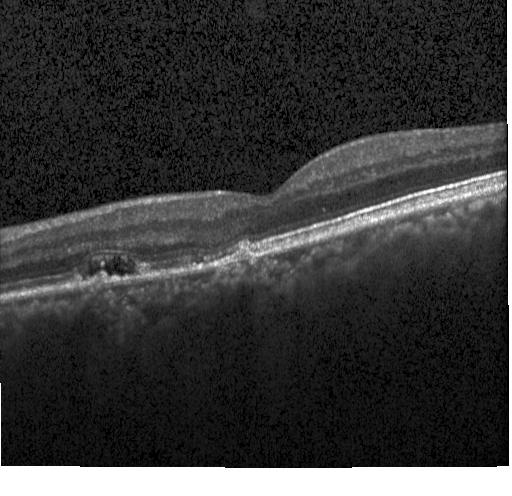

Macular scan · acquired on a Heidelberg Spectralis · optical coherence tomography B-scan — OCT finding: choroidal neovascularization (CNV).